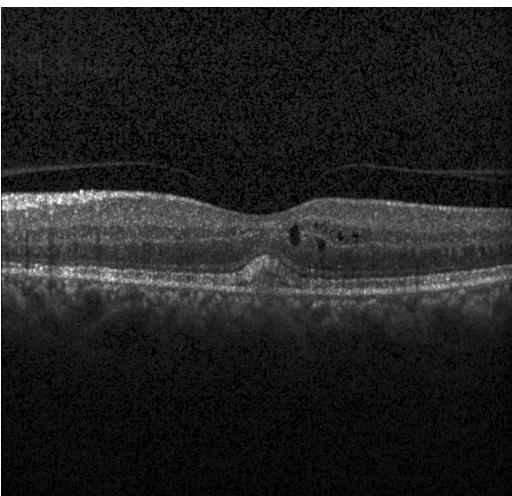

Retinal OCT cross-section showing CNV.